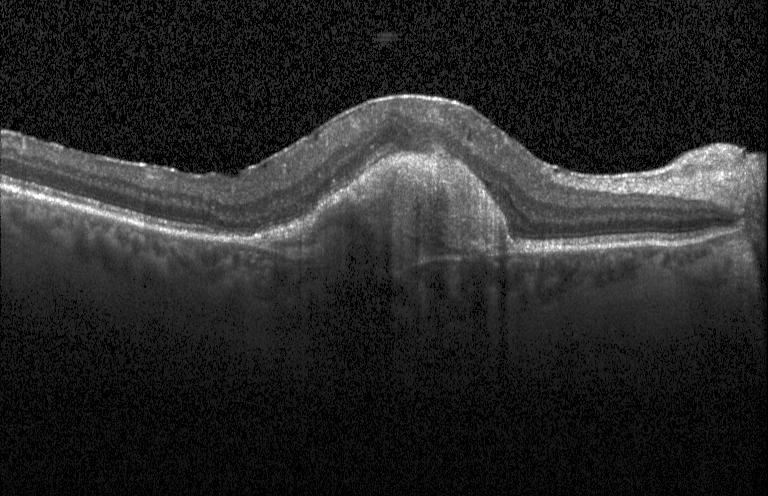
Heidelberg Spectralis. Optical coherence tomography B-scan. Horizontal scan through the fovea — Impression: choroidal neovascularization.